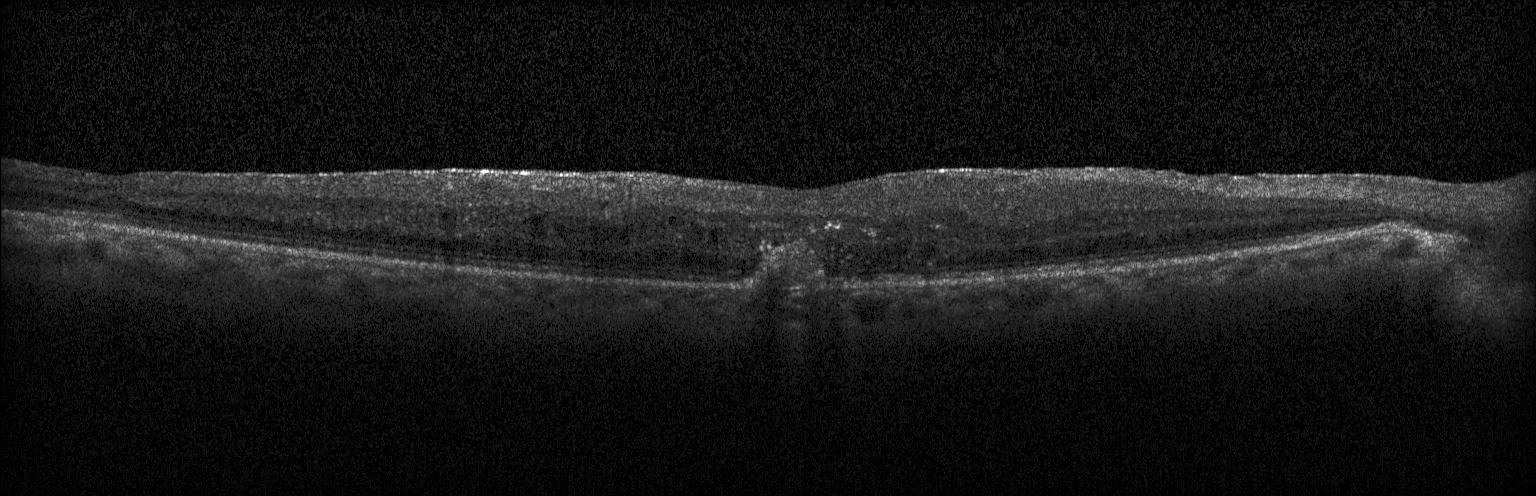
OCT B-scan.
Finding: sub-RPE drusenoid deposits.